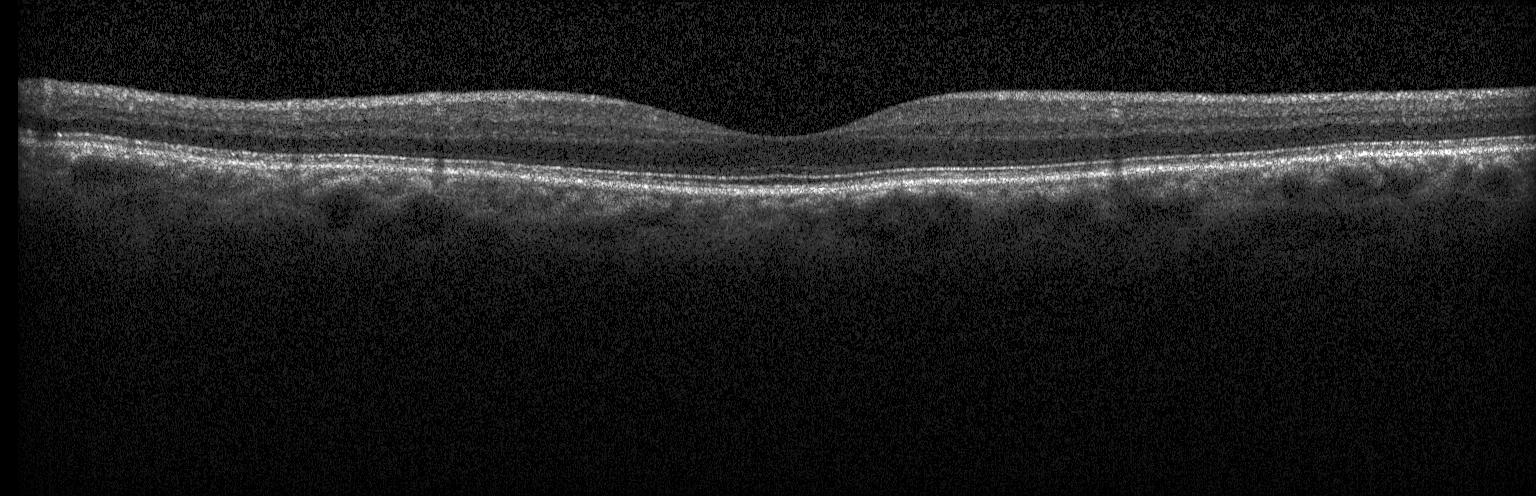
No evidence of choroidal neovascularization, diabetic macular edema, or drusen.